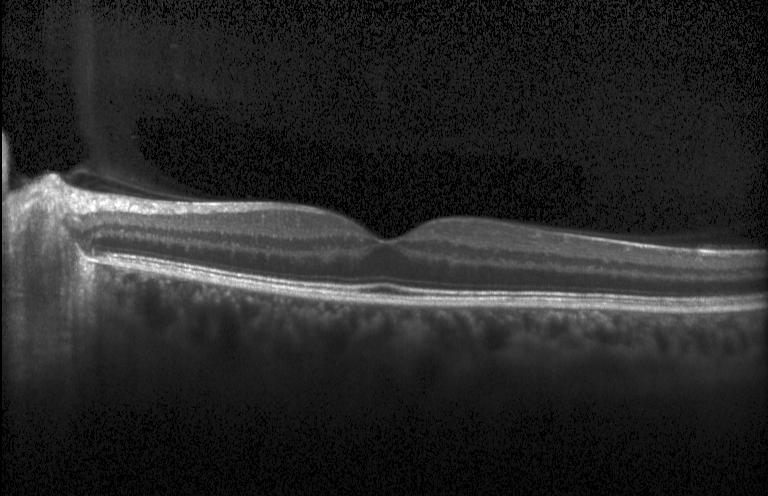

Instrument: Heidelberg Spectralis; spectral-domain OCT; OCT B-scan; through the macula — Finding: neither CNV, DME, nor drusen.